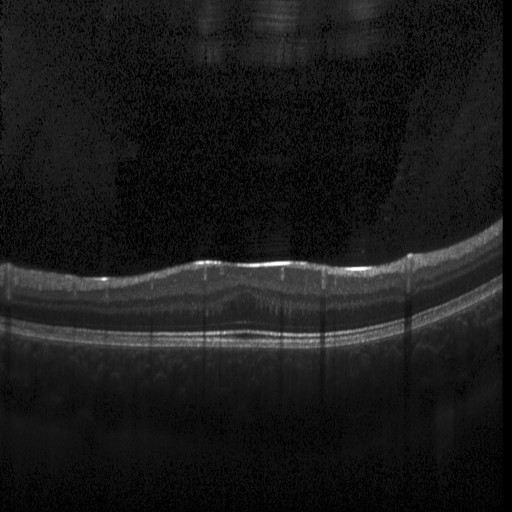
Macular OCT: diabetic macular edema (DME).